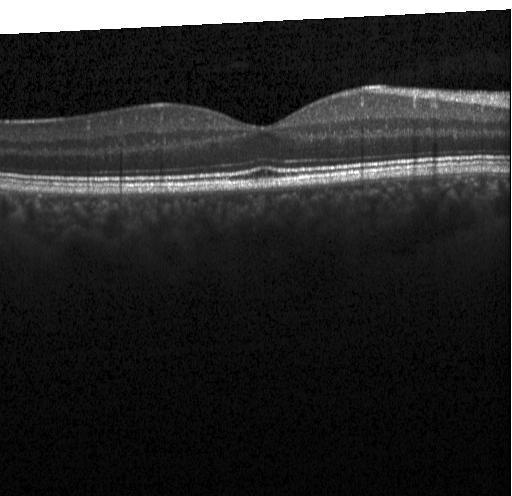
Impression: neither CNV, DME, nor drusen.